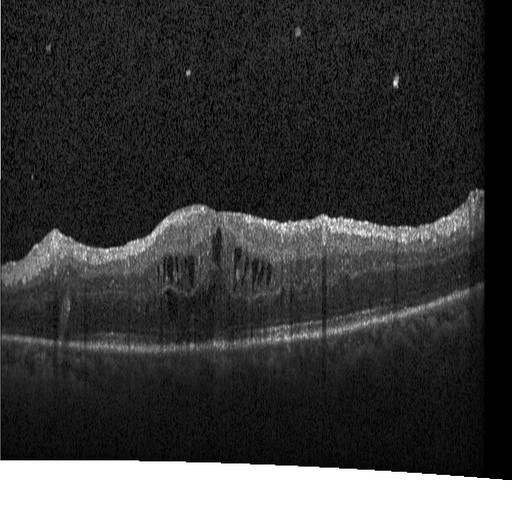 Retinal OCT cross-section showing DME.